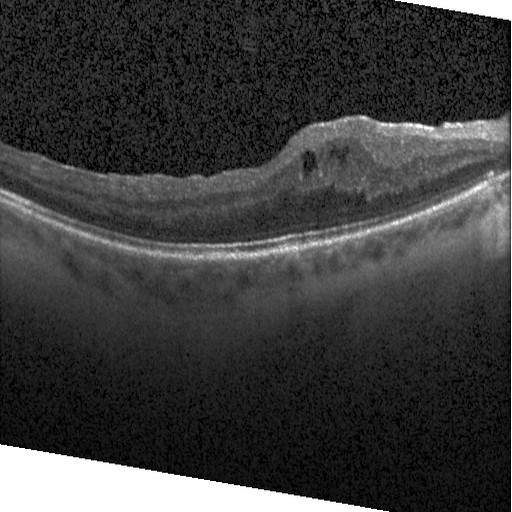

OCT B-scan · through the macula.
Diabetic macular edema (DME).